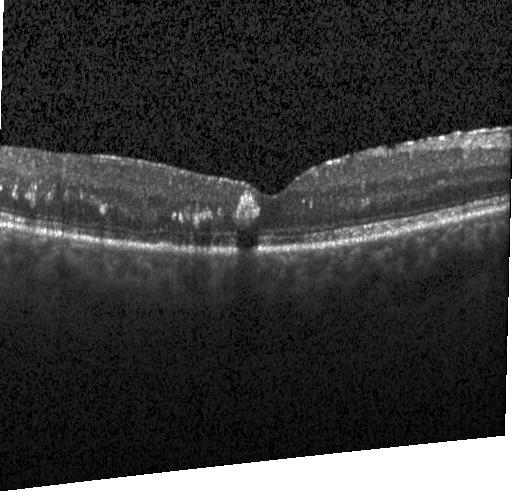

This B-scan demonstrates diabetic macular edema.